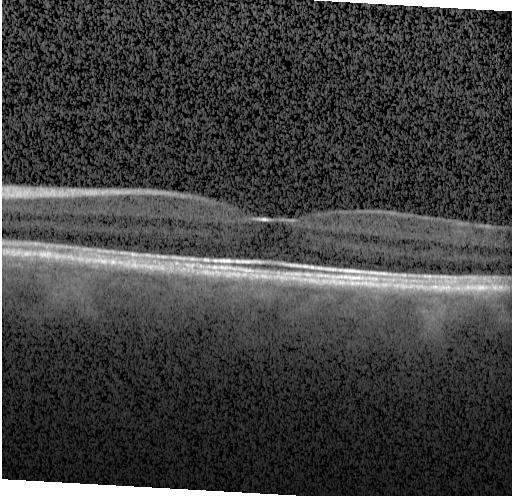
Neither choroidal neovascularization, diabetic macular edema, nor drusen.